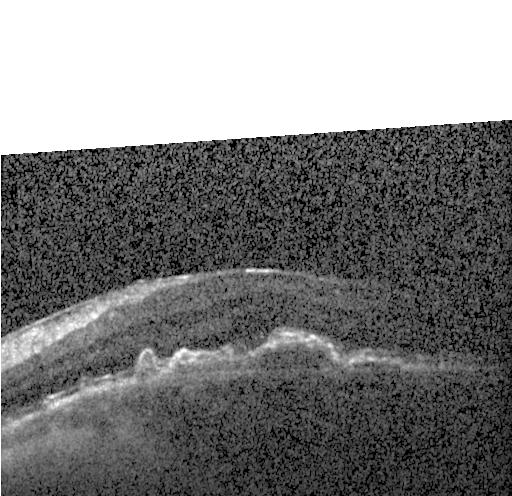
Spectral-domain optical coherence tomography. Optical coherence tomography scan. Acquired on a Heidelberg Spectralis. Through the macula
Finding: a choroidal neovascular membrane.